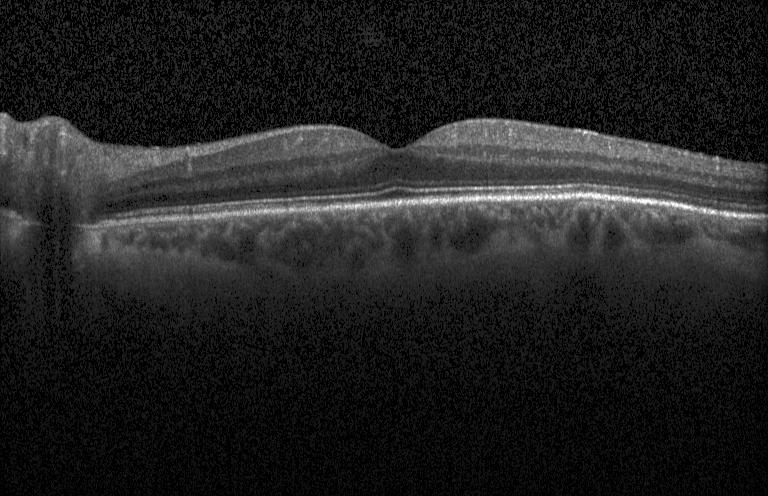
OCT line scan. Macular scan. SD-OCT. Acquired on a Heidelberg Spectralis — Diagnosis: neither choroidal neovascularization, diabetic macular edema, nor drusen.